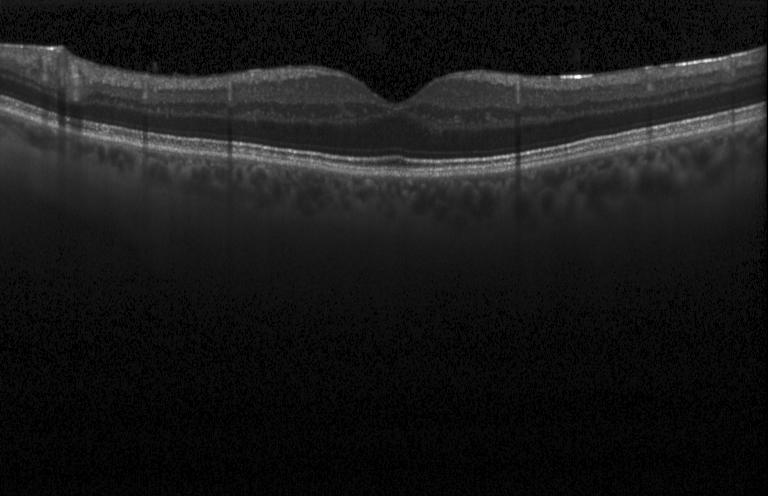
Instrument: Heidelberg Spectralis; spectral-domain OCT; retinal OCT cross-section; centered on the fovea.
Assessment: no evidence of choroidal neovascularization, diabetic macular edema, or drusen.